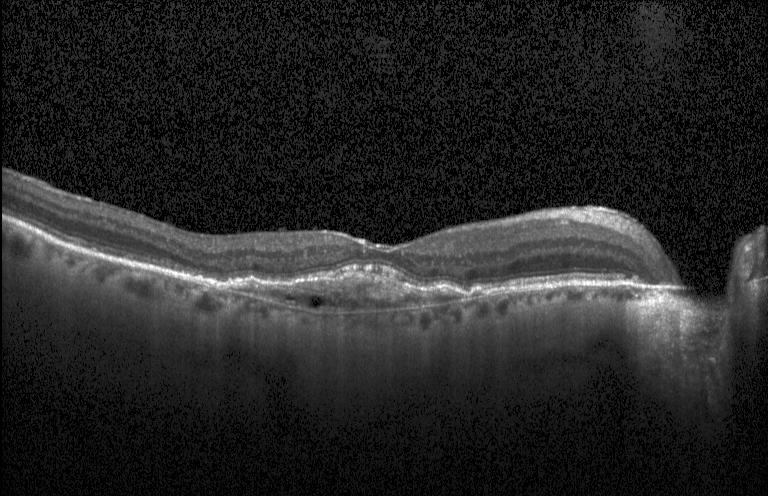

Finding: a choroidal neovascular membrane.